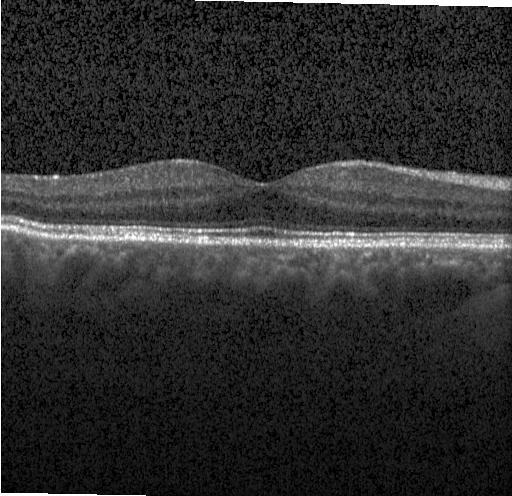
Heidelberg Spectralis OCT system · optical coherence tomography B-scan · spectral-domain OCT — Diagnosis: no CNV, no DME, and no drusen.